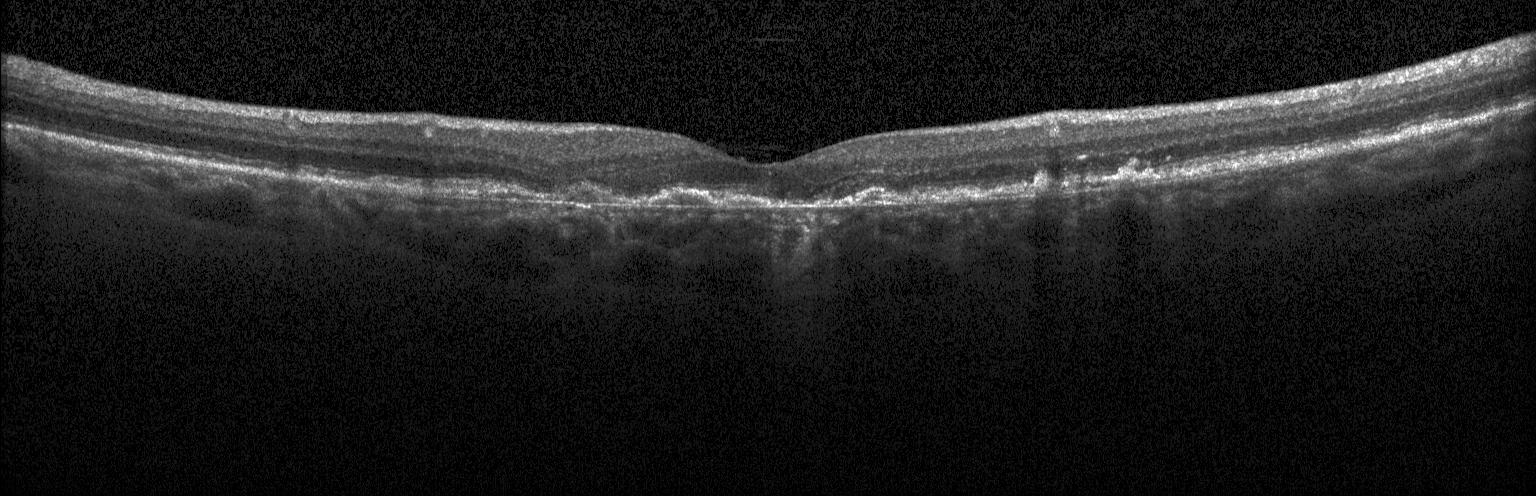

Dx: CNV.